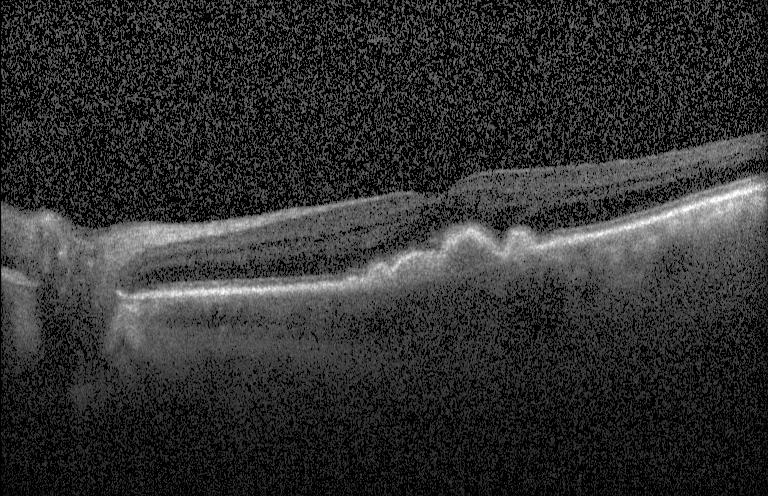

Dx: CNV.